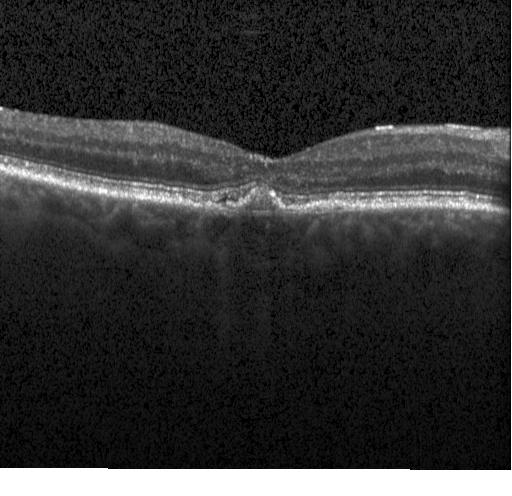

Optical coherence tomography scan; centered on the fovea; Heidelberg Spectralis OCT system; spectral-domain OCT — Finding: choroidal neovascularization (CNV).